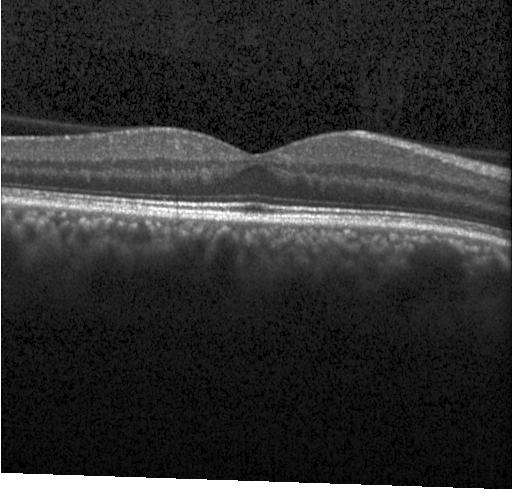

Impression: neither choroidal neovascularization, diabetic macular edema, nor drusen.